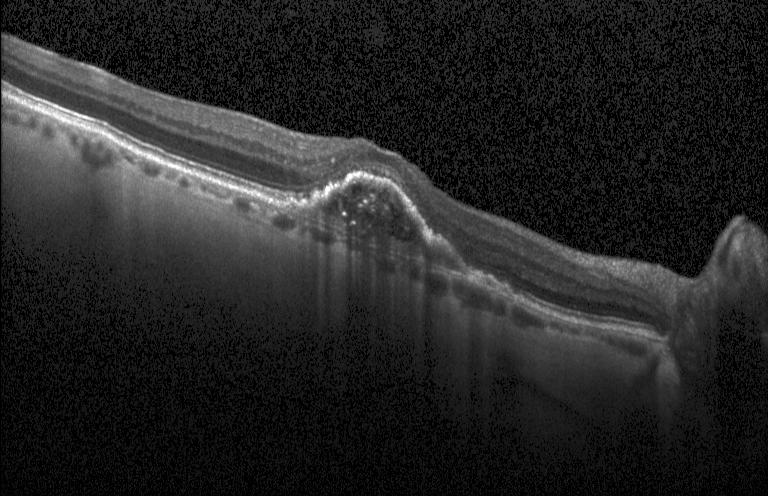 Macular OCT: a choroidal neovascular membrane.